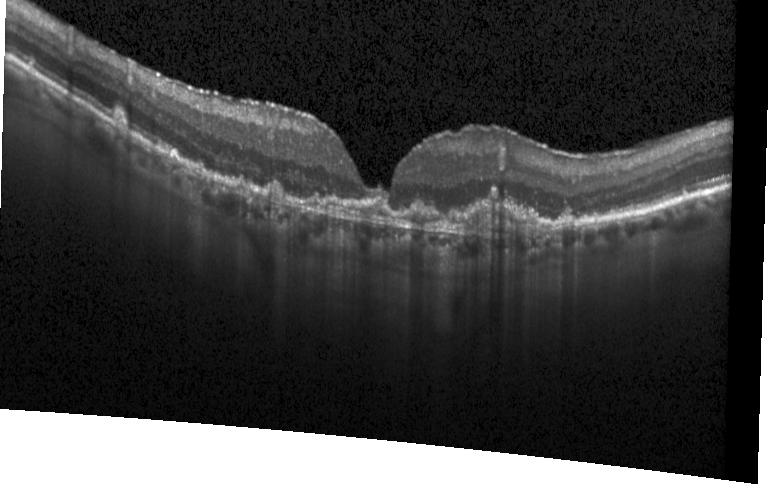
Finding: CNV.